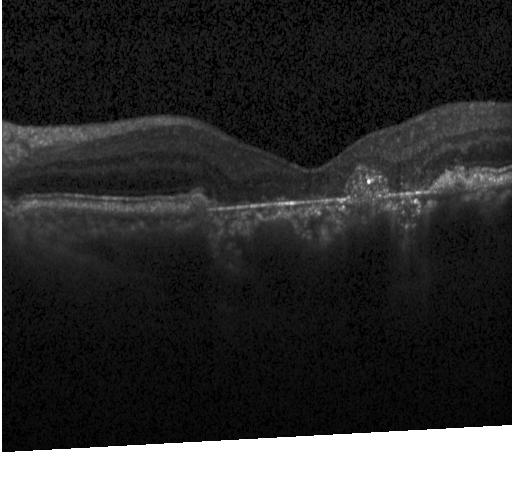

OCT line scan — OCT finding: CNV.